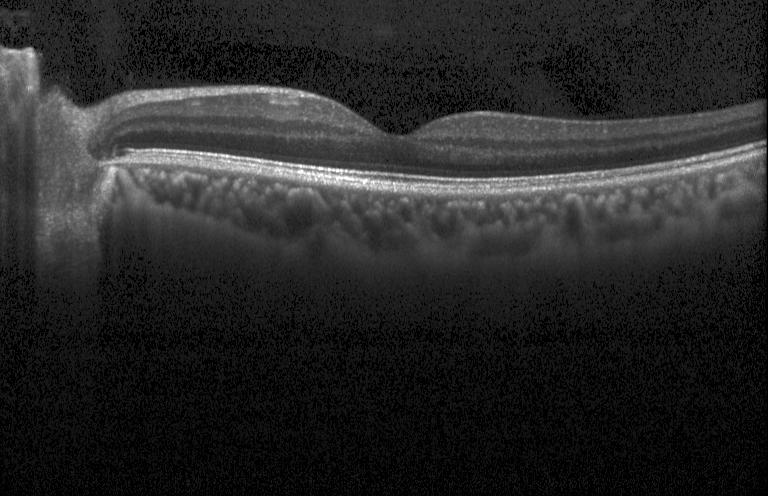

Spectral-domain optical coherence tomography. Heidelberg Spectralis OCT system. Fovea-centered. OCT B-scan
OCT finding: no evidence of choroidal neovascularization, diabetic macular edema, or drusen.